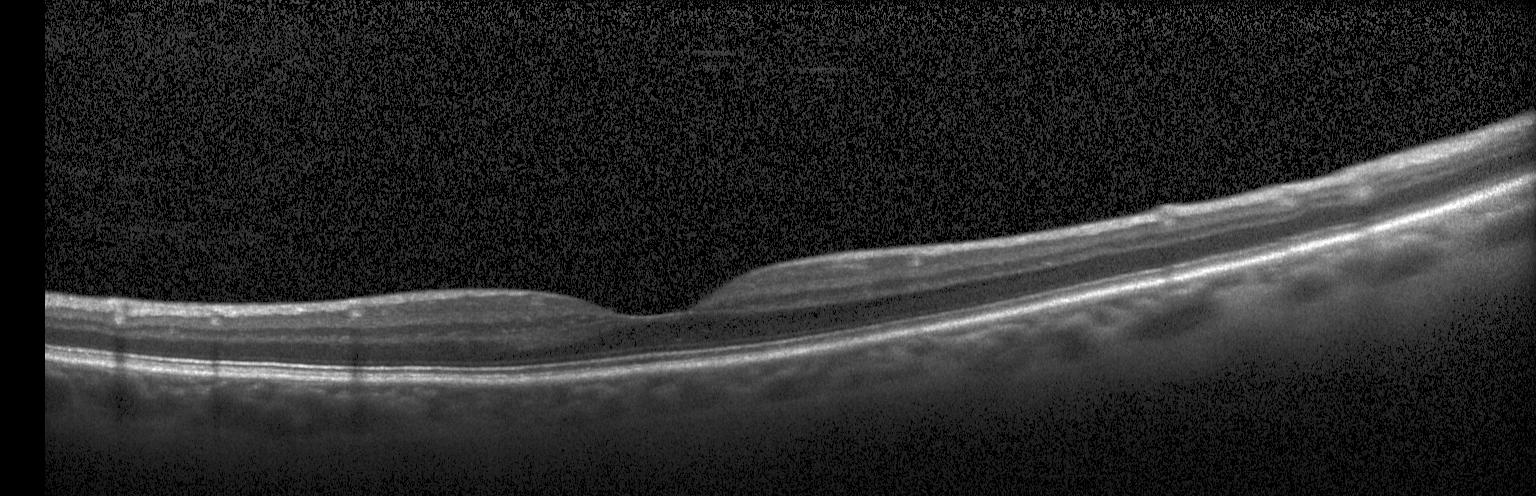
Optical coherence tomography B-scan, horizontal scan through the fovea — The scan shows no evidence of CNV, DME, or drusen.